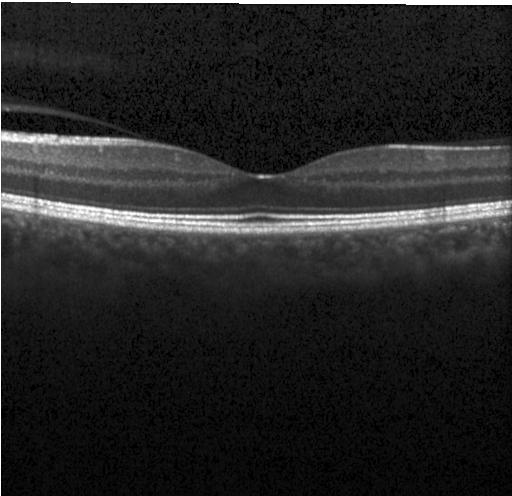

Assessment: no choroidal neovascularization, no diabetic macular edema, and no drusen.